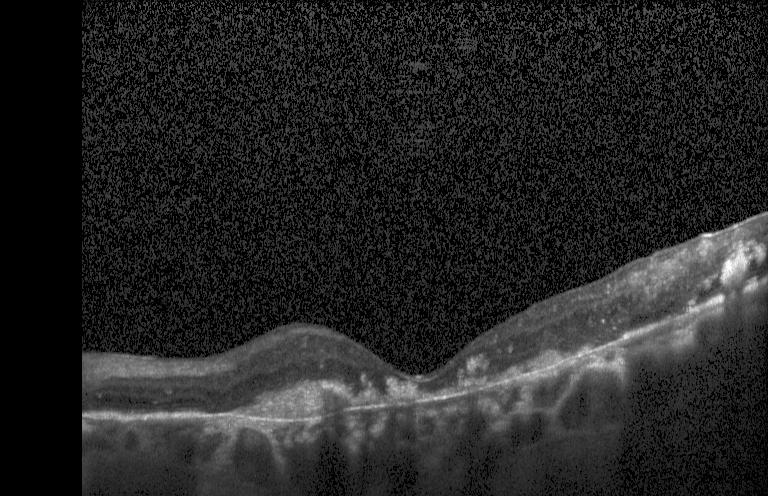
OCT B-scan showing a choroidal neovascular membrane.